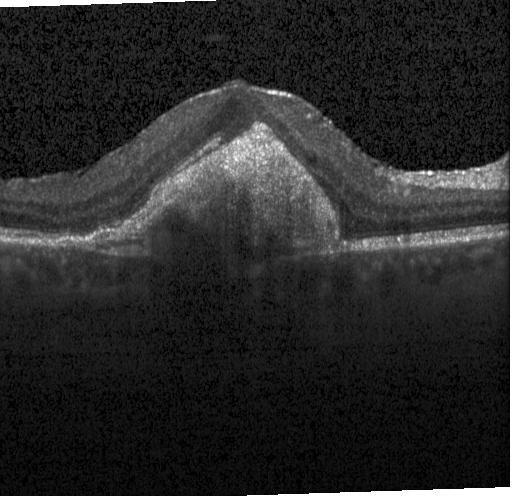
Heidelberg Spectralis; OCT B-scan
Diagnosis: a choroidal neovascular membrane.